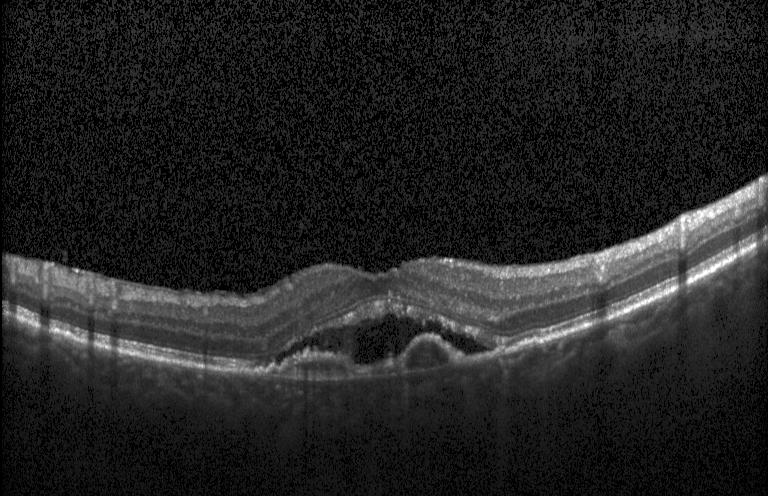
OCT line scan, SD-OCT, Heidelberg Spectralis
CNV.